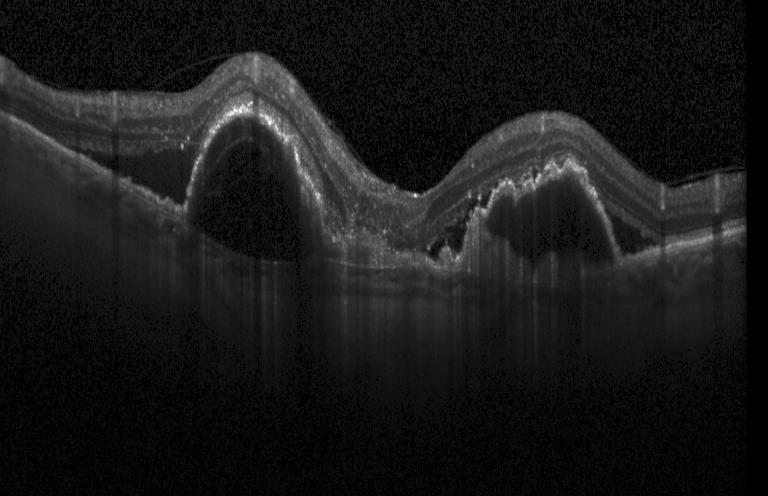
OCT B-scan. SD-OCT. Heidelberg Spectralis.
This B-scan demonstrates a choroidal neovascular membrane.